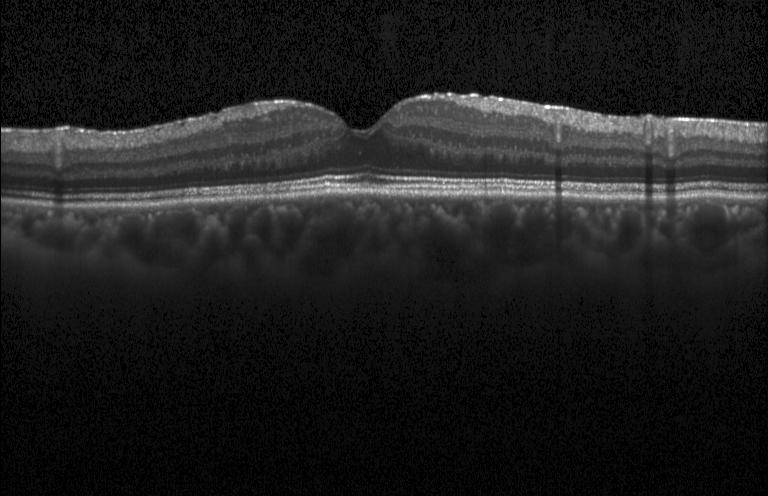 Retinal OCT cross-section showing no choroidal neovascularization, diabetic macular edema, or drusen.